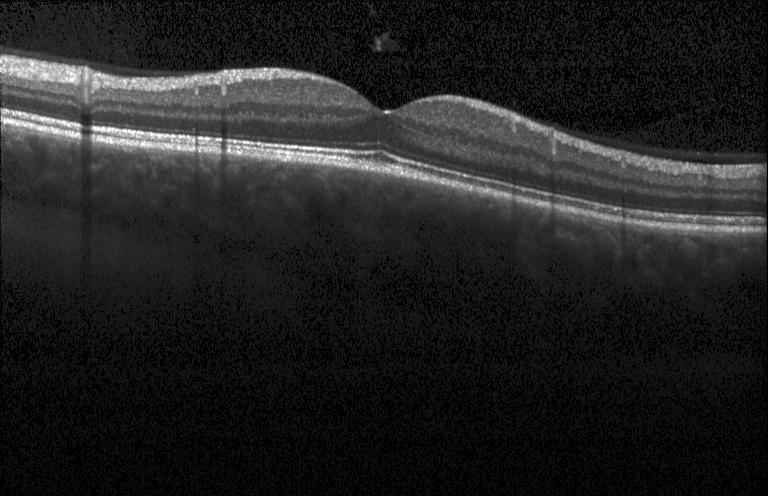

Heidelberg Spectralis OCT system, fovea-centered, spectral-domain OCT, optical coherence tomography scan — OCT finding: neither choroidal neovascularization, diabetic macular edema, nor drusen.